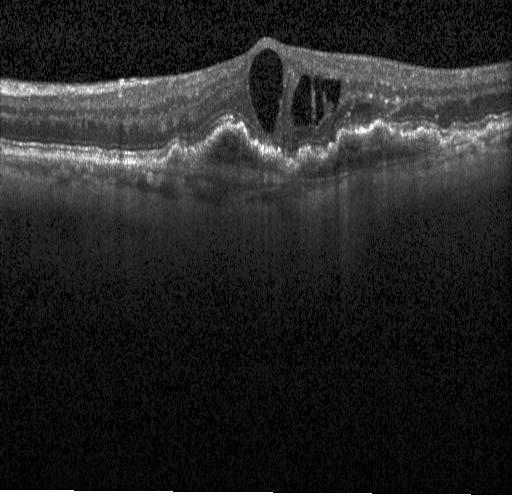

Optical coherence tomography B-scan · SD-OCT. Choroidal neovascularization (CNV).